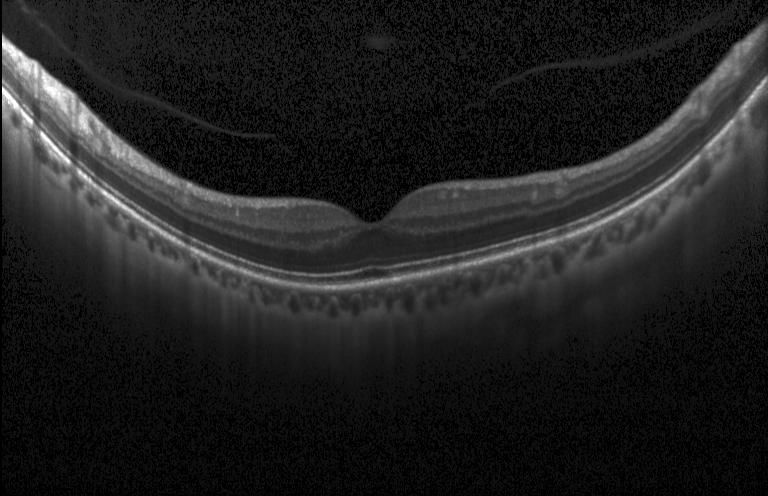 This B-scan demonstrates neither CNV, DME, nor drusen.